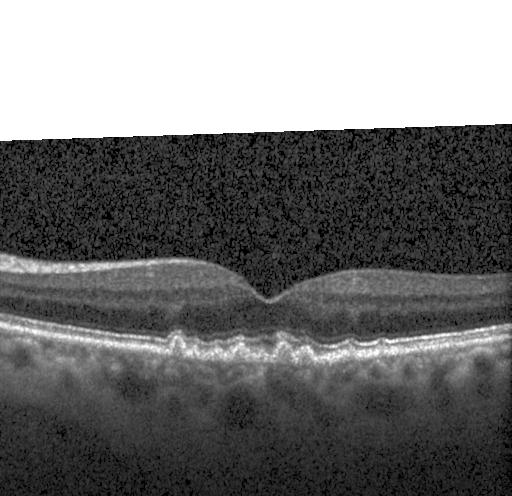 Finding: sub-RPE drusenoid deposits.